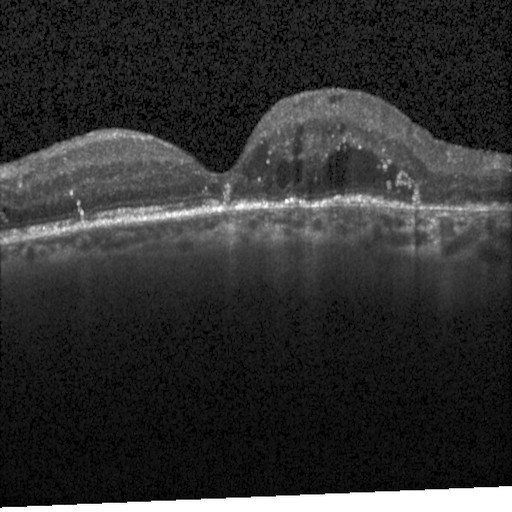

Spectral-domain OCT; retinal OCT cross-section — This B-scan demonstrates DME.